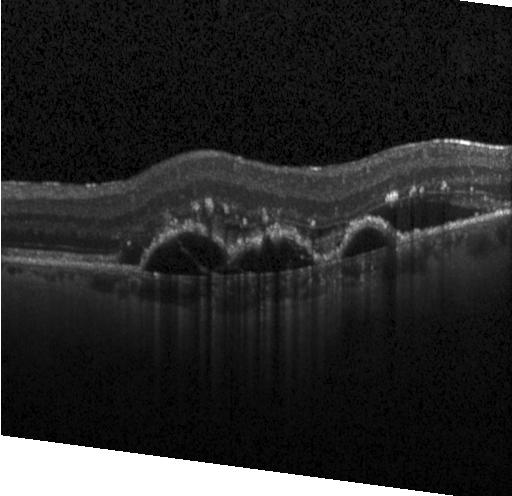

Heidelberg Spectralis. Spectral-domain optical coherence tomography. Optical coherence tomography scan. Through the macula
Diagnosis: choroidal neovascularization (CNV).